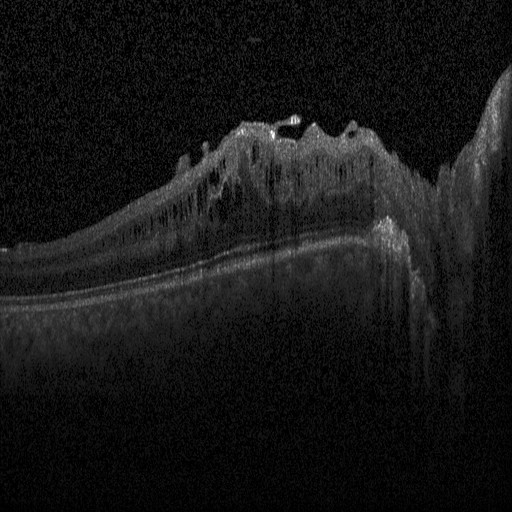 Macular OCT: DME.